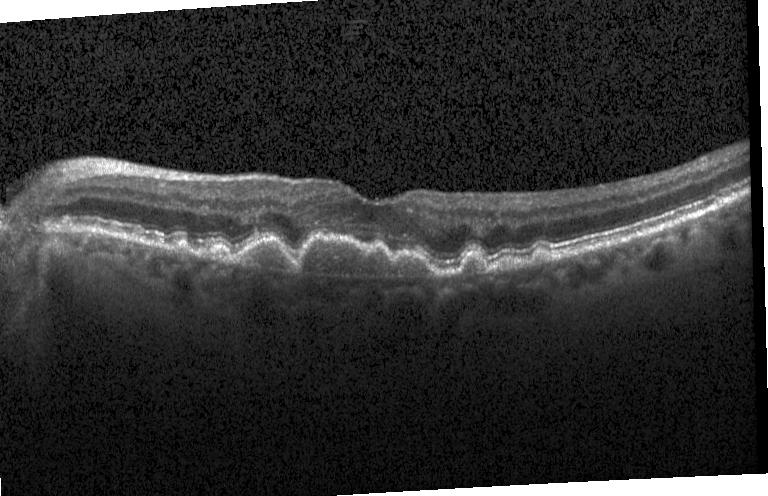
Finding: CNV.